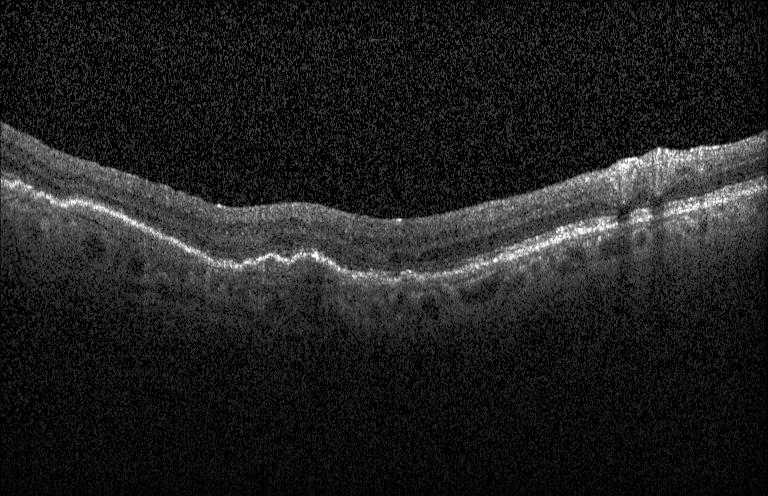

Optical coherence tomography B-scan. Acquired on a Heidelberg Spectralis — A choroidal neovascular membrane.